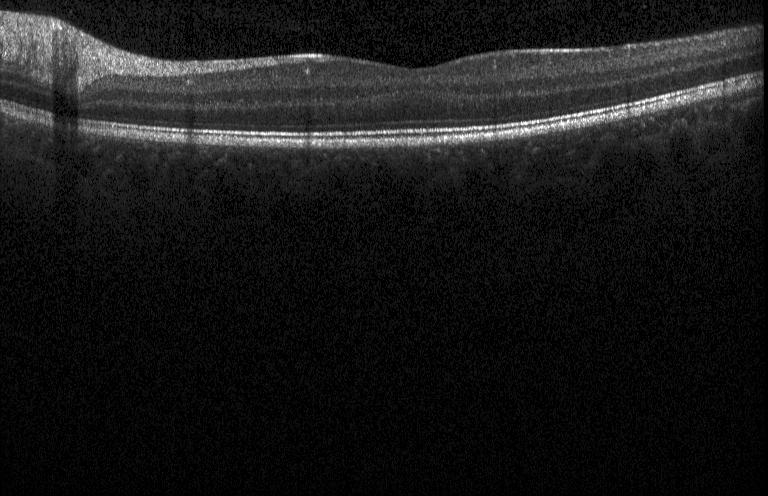

This B-scan demonstrates no evidence of choroidal neovascularization, diabetic macular edema, or drusen.